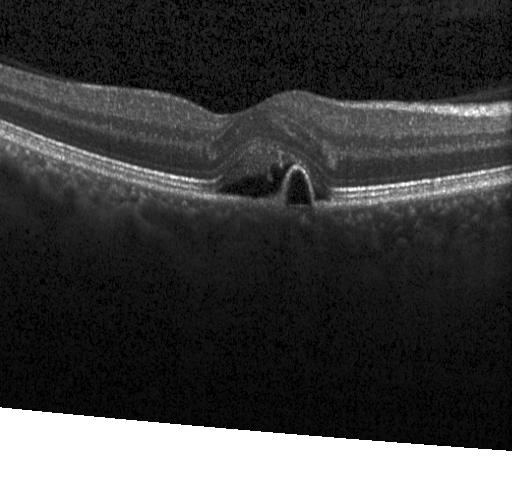
Finding: a choroidal neovascular membrane.